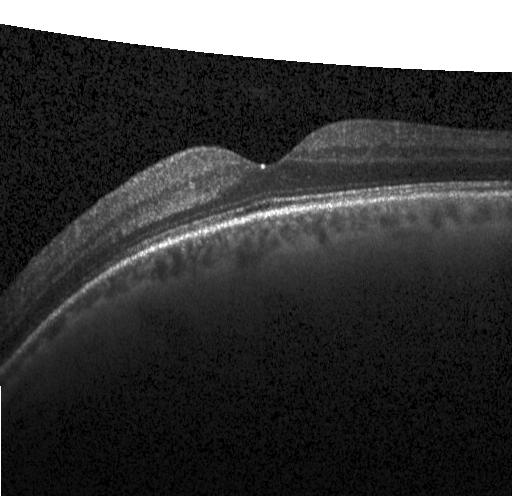
Retinal OCT B-scan · fovea-centered · SD-OCT · Heidelberg Spectralis OCT system. Macular OCT: no evidence of choroidal neovascularization, diabetic macular edema, or drusen.